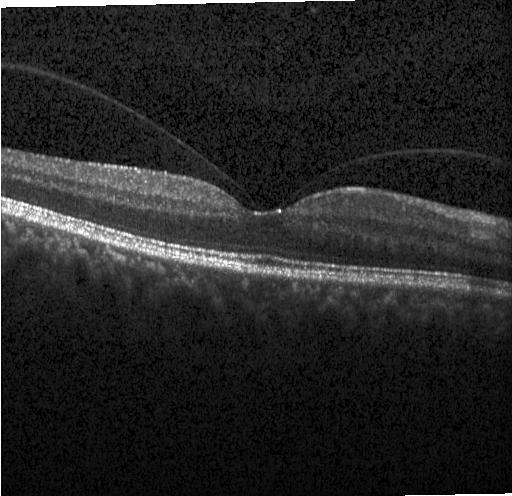
Heidelberg Spectralis. OCT line scan — Diagnosis: no CNV, DME, or drusen.